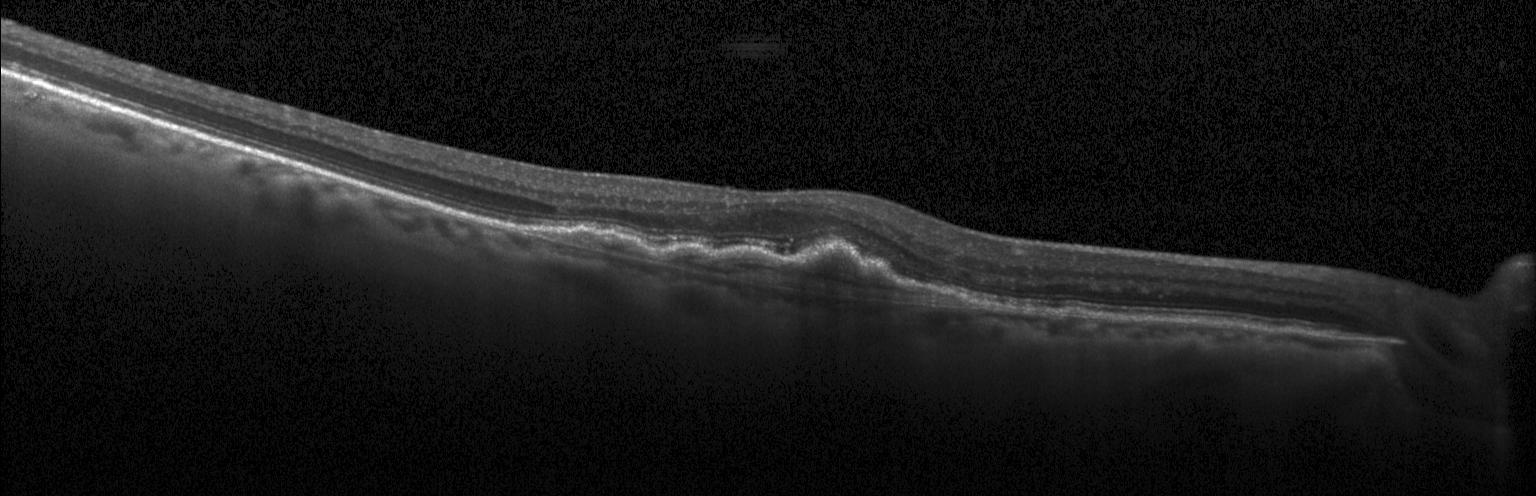
Optical coherence tomography B-scan — Macular OCT: a choroidal neovascular membrane.